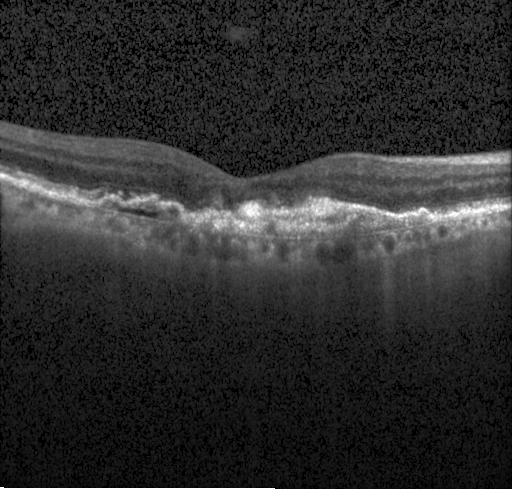 Retinal OCT B-scan — The scan shows choroidal neovascularization.